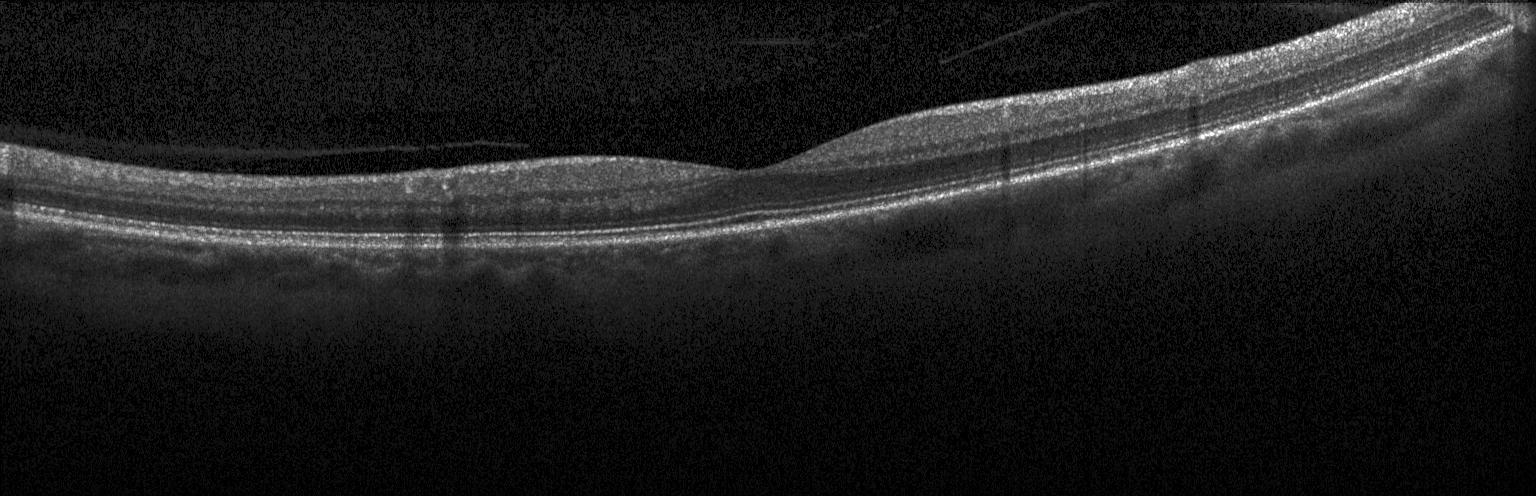
Heidelberg Spectralis OCT system. Through the macula. Spectral-domain optical coherence tomography. Optical coherence tomography scan.
Finding: neither choroidal neovascularization, diabetic macular edema, nor drusen.